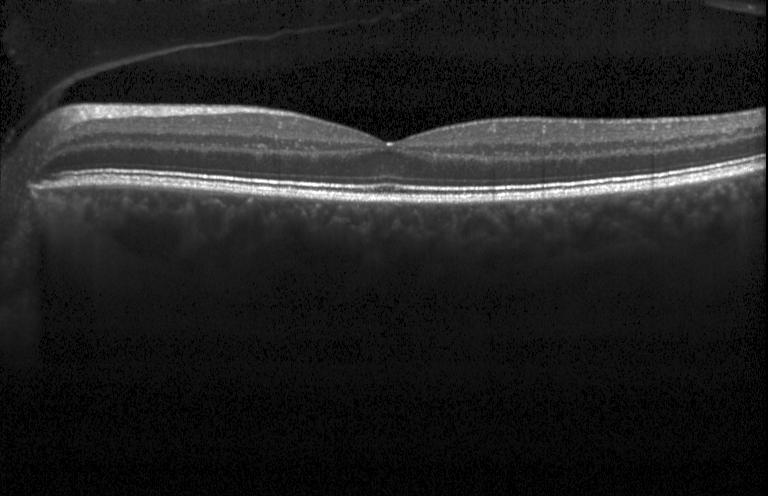
Through the macula. Retinal OCT cross-section. SD-OCT — Impression: no CNV, no DME, and no drusen.